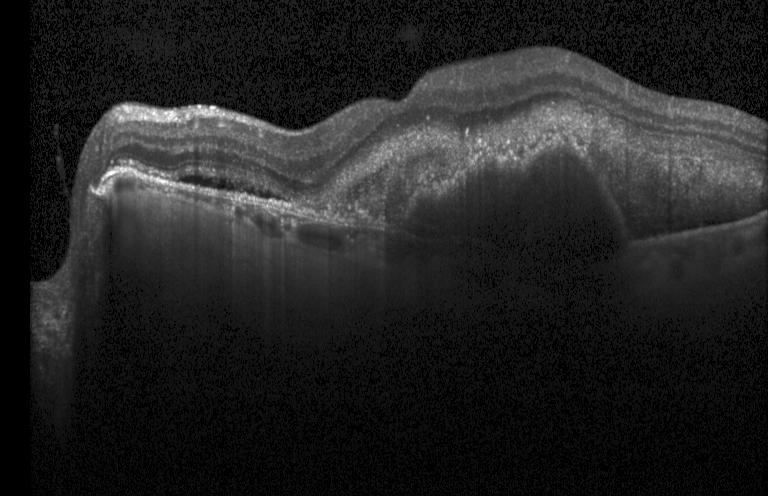

Macular OCT: choroidal neovascularization (CNV).